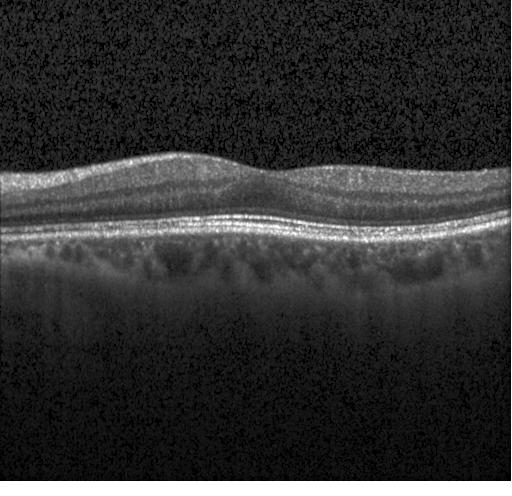

Horizontal scan through the fovea; acquired on a Heidelberg Spectralis; OCT line scan. The scan shows no choroidal neovascularization, diabetic macular edema, or drusen.